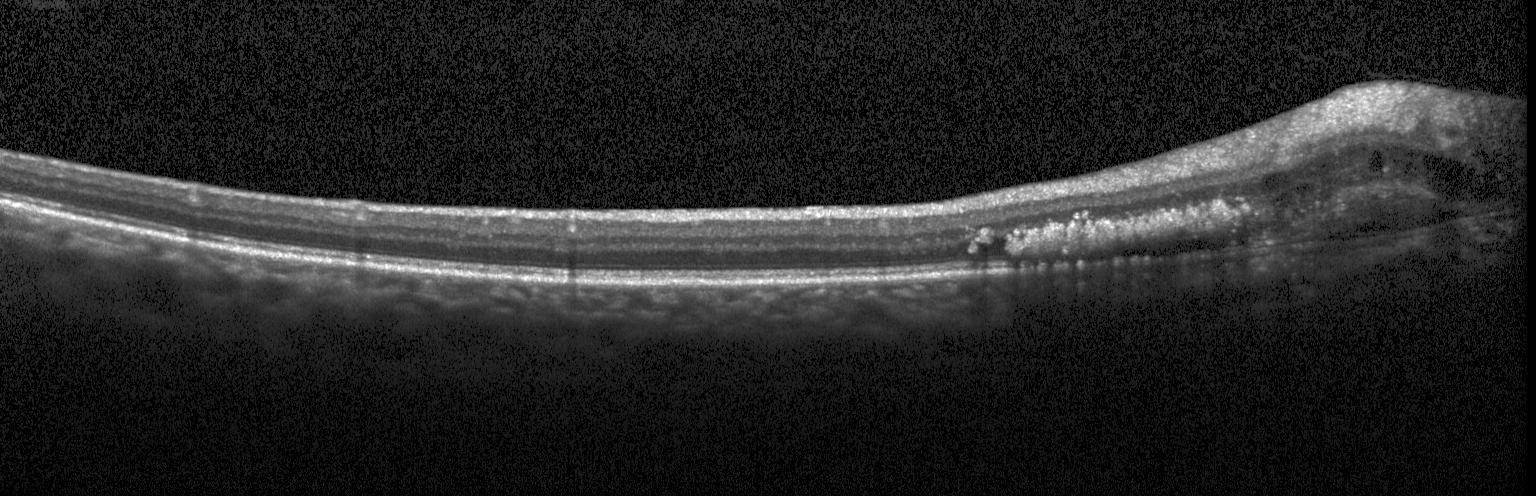
OCT line scan, fovea-centered
The scan shows a choroidal neovascular membrane.